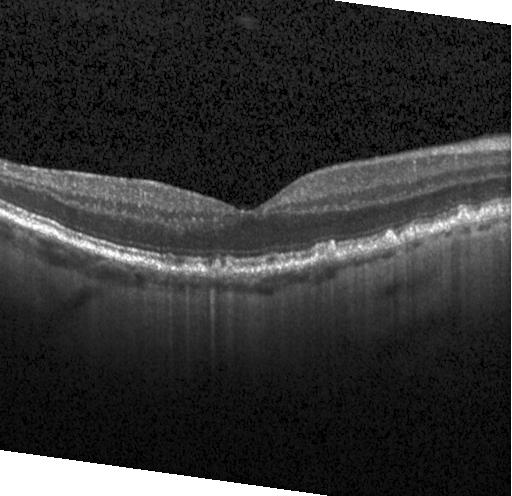 Impression: sub-RPE drusenoid deposits.